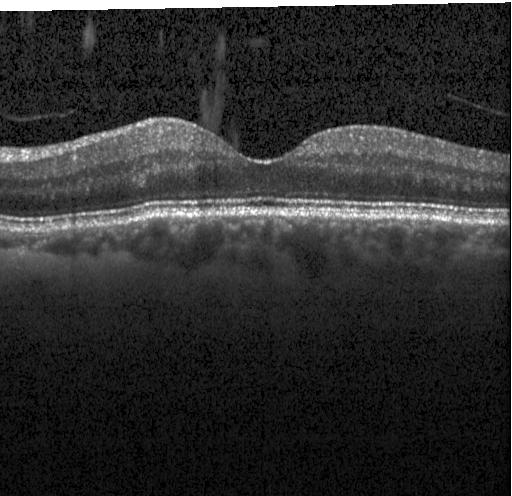 Retinal OCT B-scan — Impression: no evidence of choroidal neovascularization, diabetic macular edema, or drusen.